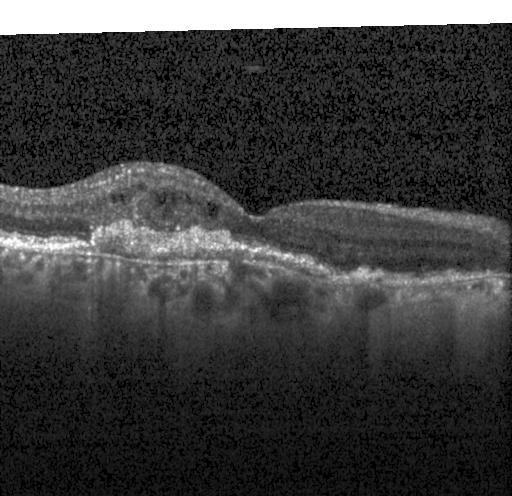 Impression: CNV.